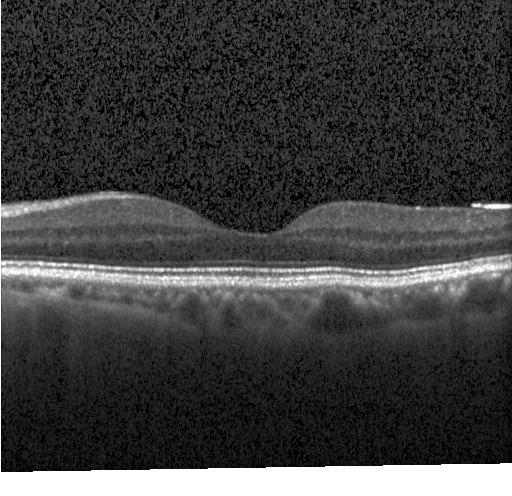 Spectral-domain optical coherence tomography; Heidelberg Spectralis; optical coherence tomography scan.
Neither CNV, DME, nor drusen.